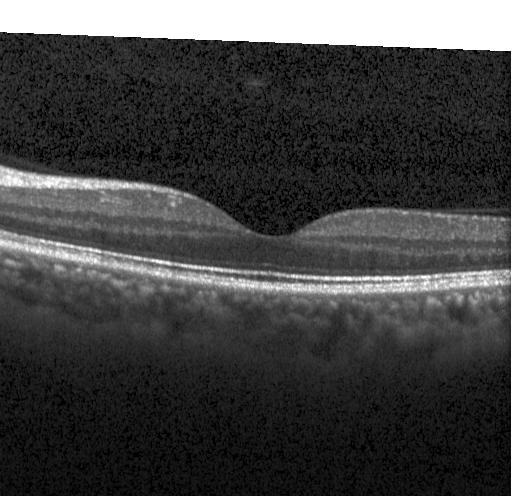 Optical coherence tomography scan; Heidelberg Spectralis; centered on the fovea
Macular OCT: neither CNV, DME, nor drusen.